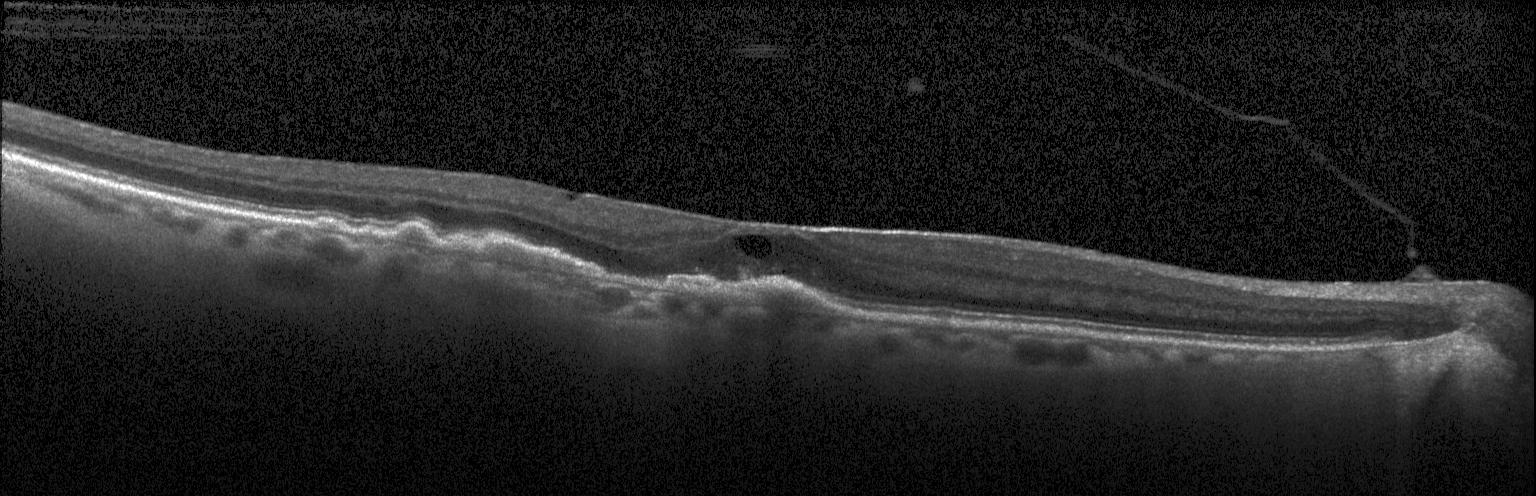

Diagnosis: choroidal neovascularization.